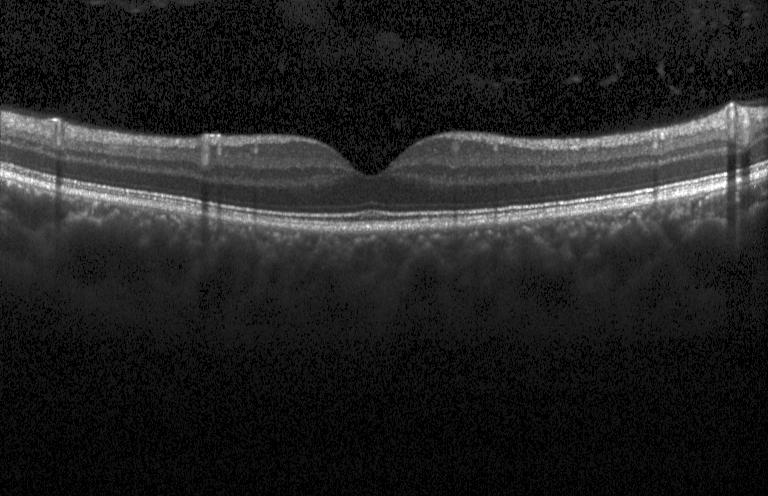 Diagnosis: no choroidal neovascularization, diabetic macular edema, or drusen.